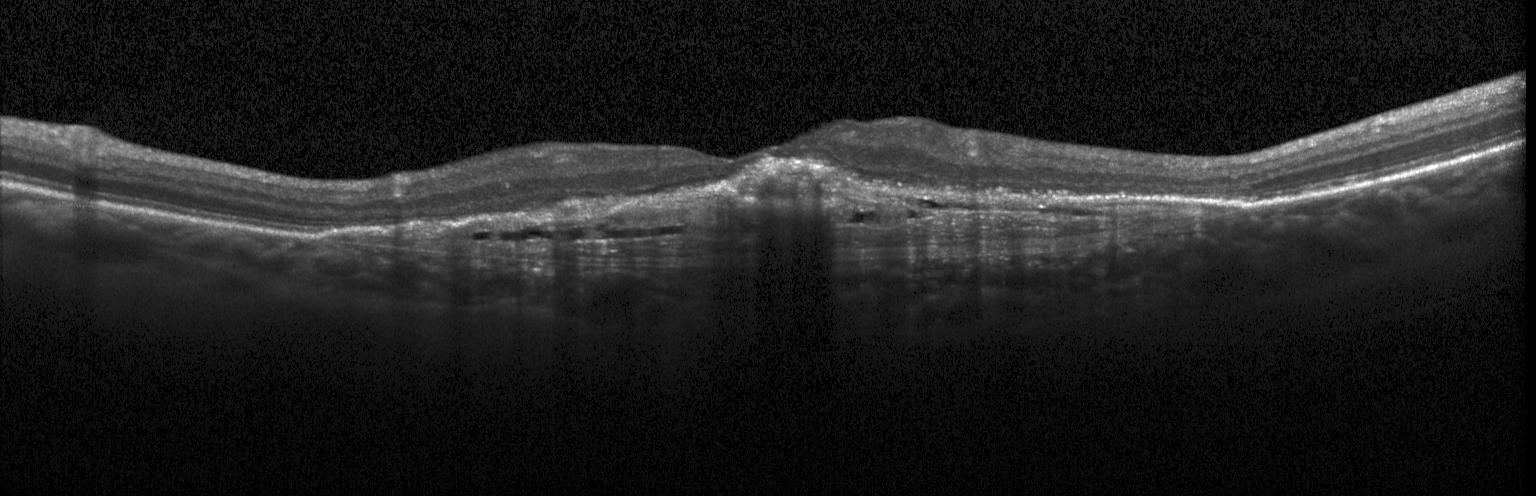 SD-OCT, centered on the fovea, OCT line scan, Heidelberg Spectralis OCT system. This B-scan demonstrates choroidal neovascularization.